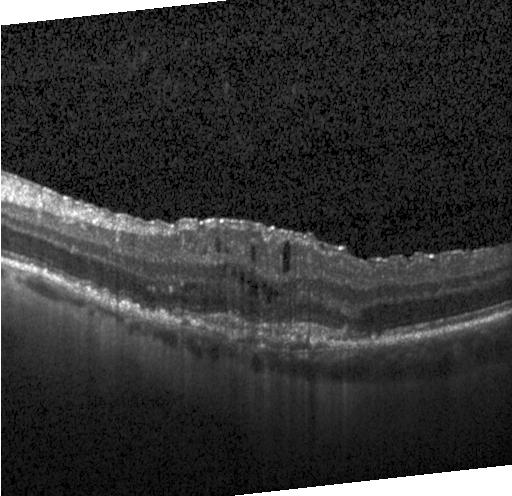

Acquired on a Heidelberg Spectralis. Retinal OCT B-scan. Spectral-domain OCT. Macular scan. Finding: a choroidal neovascular membrane.